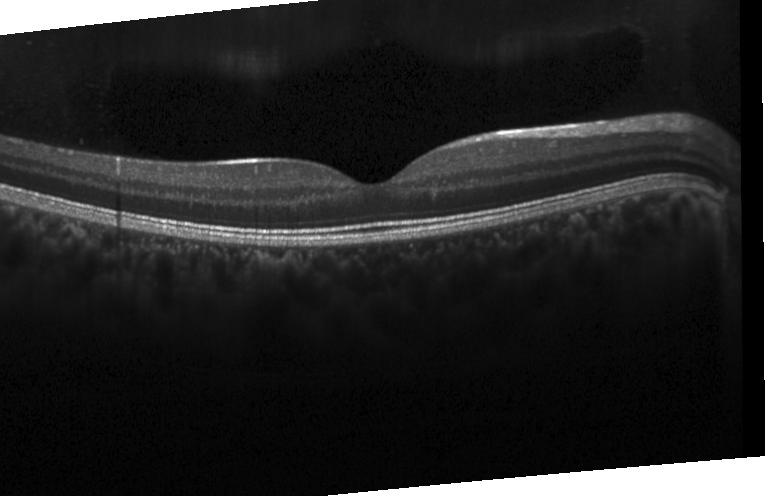

Impression: no evidence of choroidal neovascularization, diabetic macular edema, or drusen.